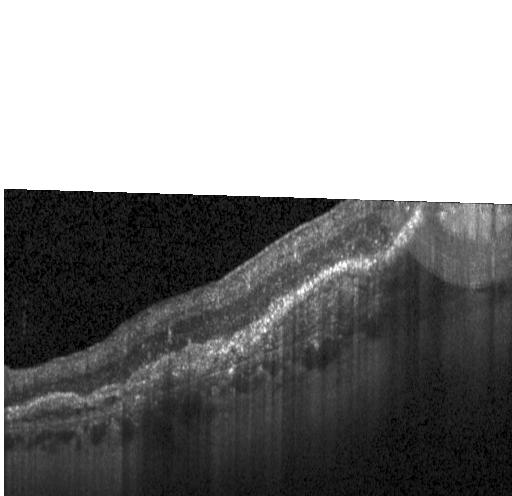 Impression: a choroidal neovascular membrane.